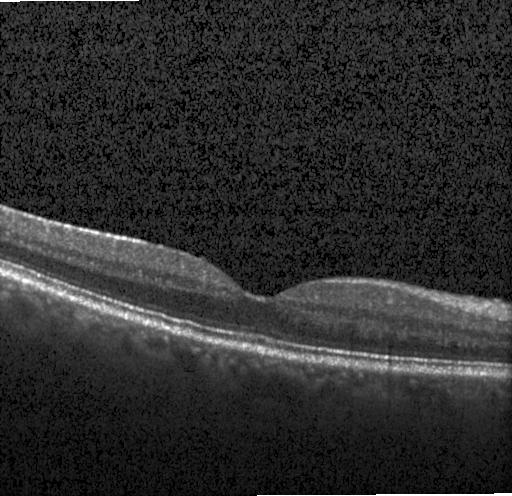

Through the macula. Retinal OCT B-scan. SD-OCT. Heidelberg Spectralis OCT system
Diagnosis: neither choroidal neovascularization, diabetic macular edema, nor drusen.